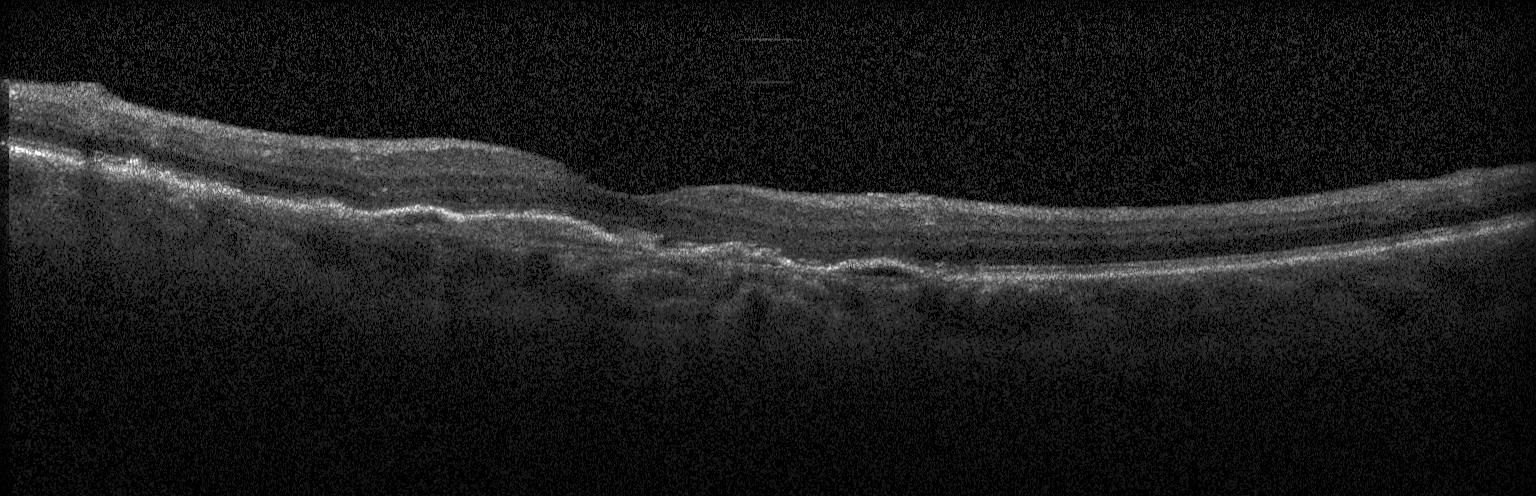
The scan shows a choroidal neovascular membrane.